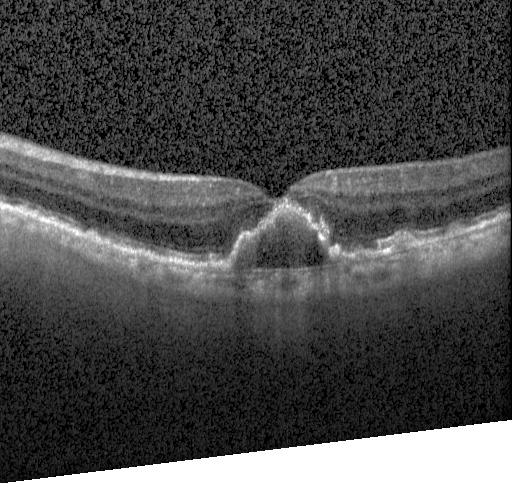
Instrument: Heidelberg Spectralis; SD-OCT; macular scan; OCT line scan.
The scan shows a choroidal neovascular membrane.